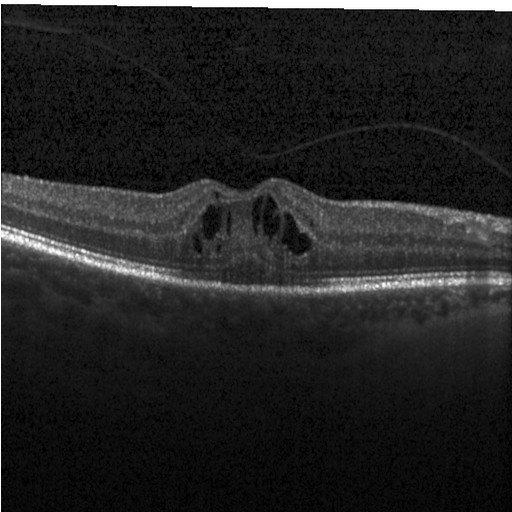
Through the macula · optical coherence tomography B-scan · Heidelberg Spectralis OCT system · spectral-domain OCT. The scan shows DME.